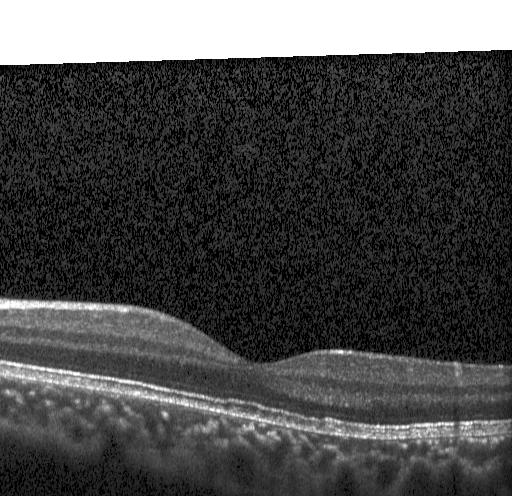 No evidence of choroidal neovascularization, diabetic macular edema, or drusen.